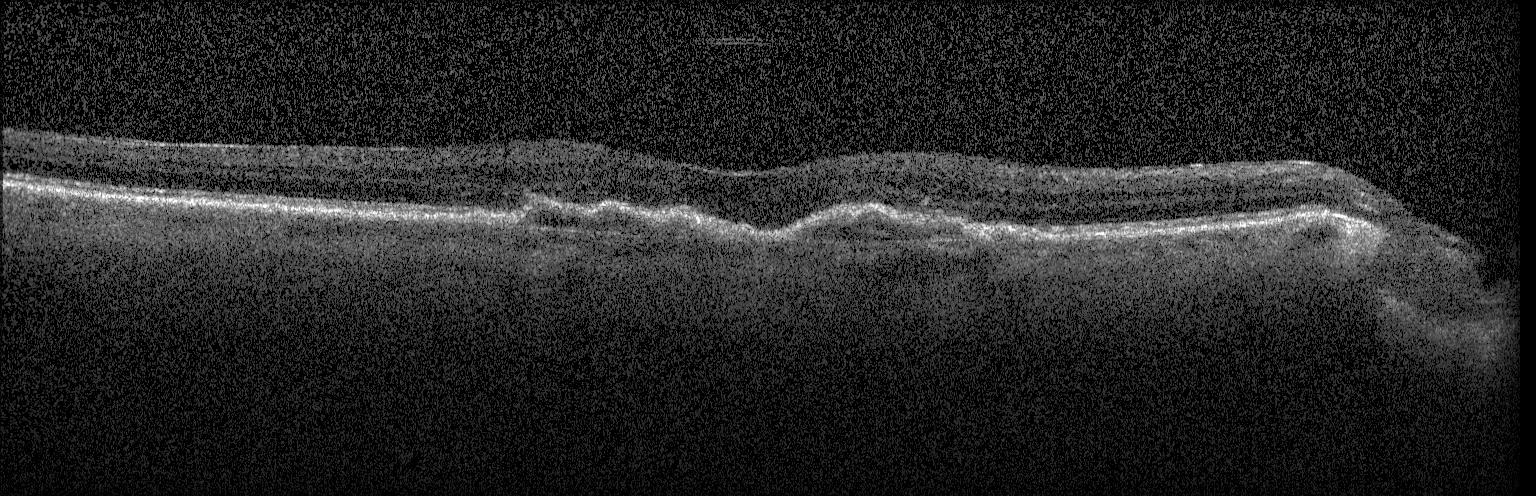
Fovea-centered; OCT line scan; spectral-domain optical coherence tomography. Impression: a choroidal neovascular membrane.